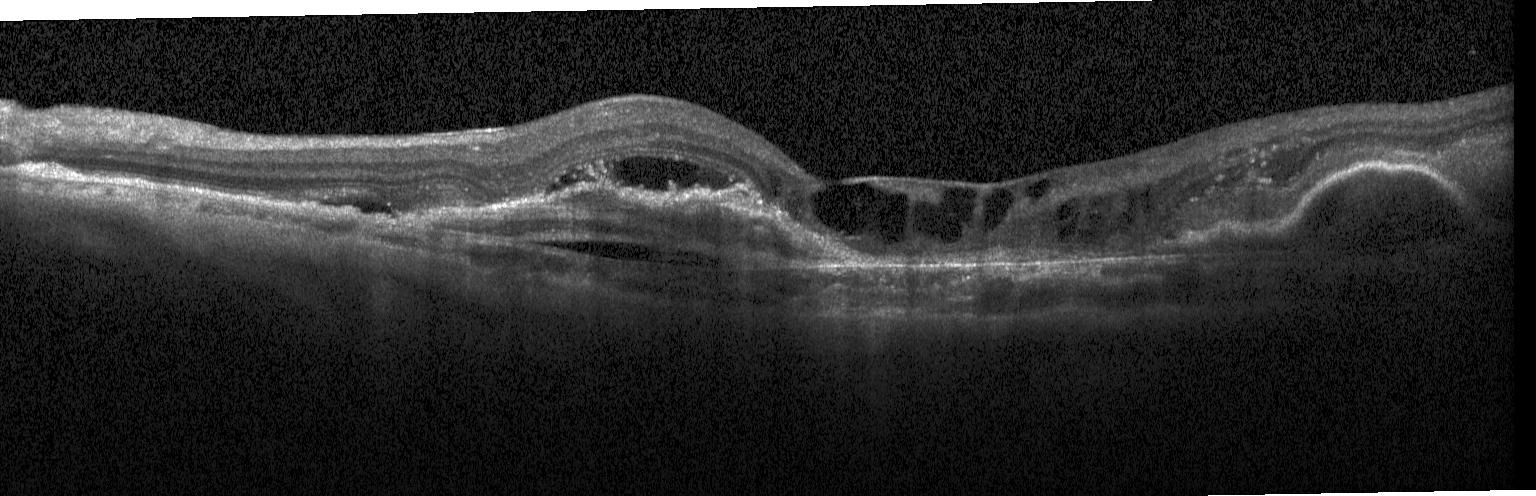 Finding: choroidal neovascularization.